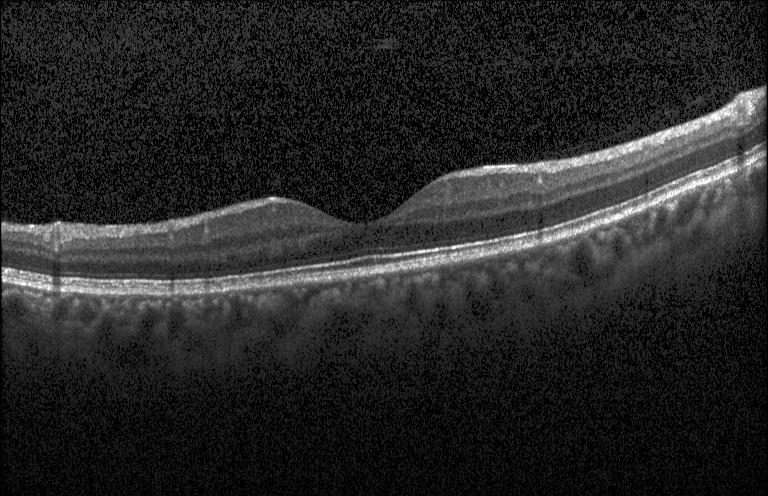

Instrument: Heidelberg Spectralis. Spectral-domain OCT. Retinal OCT cross-section. Fovea-centered. Dx: neither choroidal neovascularization, diabetic macular edema, nor drusen.